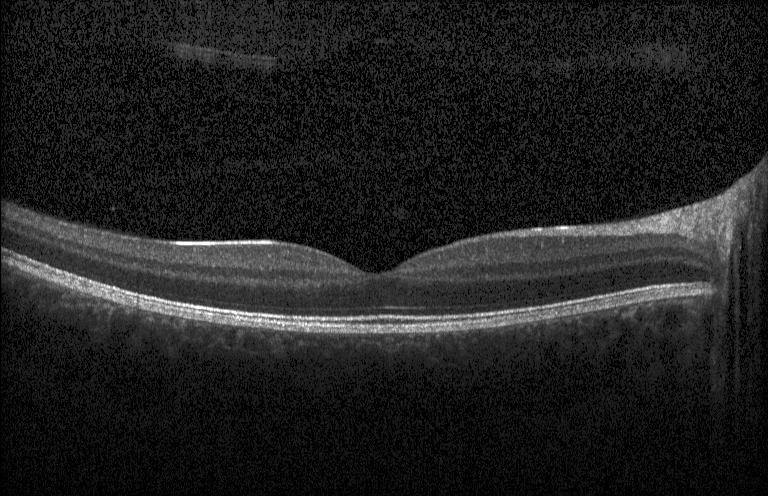
Retinal OCT cross-section, spectral-domain OCT — Finding: no CNV, no DME, and no drusen.